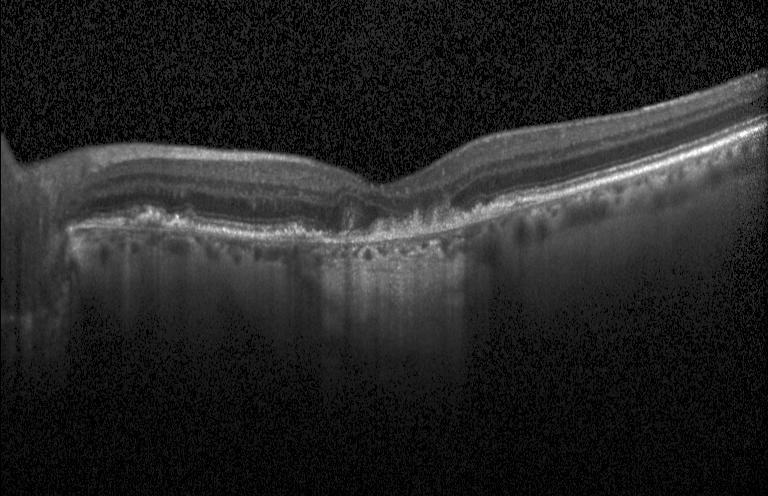

Diagnosis: a choroidal neovascular membrane.